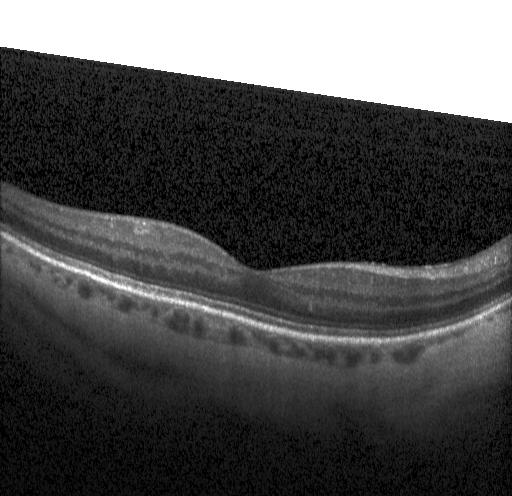

Instrument: Heidelberg Spectralis, optical coherence tomography scan, SD-OCT, fovea-centered — Finding: neither choroidal neovascularization, diabetic macular edema, nor drusen.